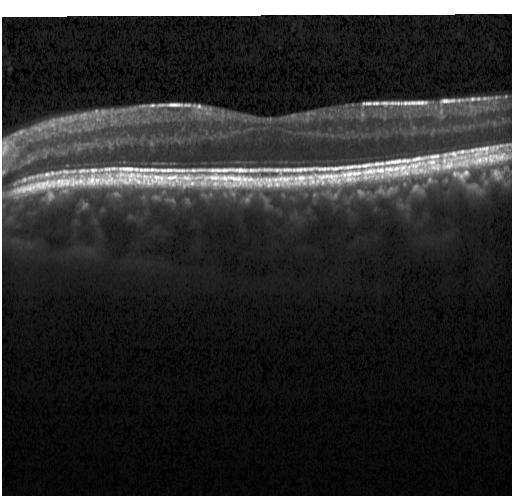

OCT line scan · instrument: Heidelberg Spectralis · SD-OCT.
Finding: no evidence of CNV, DME, or drusen.